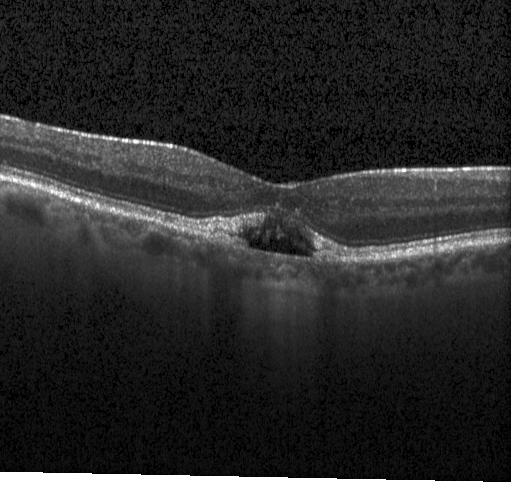 Retinal OCT cross-section. Centered on the fovea.
Diagnosis: CNV.